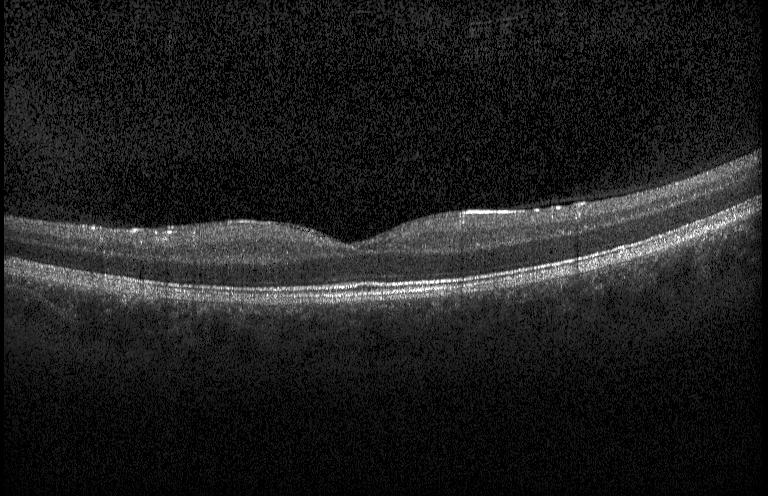 Neither choroidal neovascularization, diabetic macular edema, nor drusen.